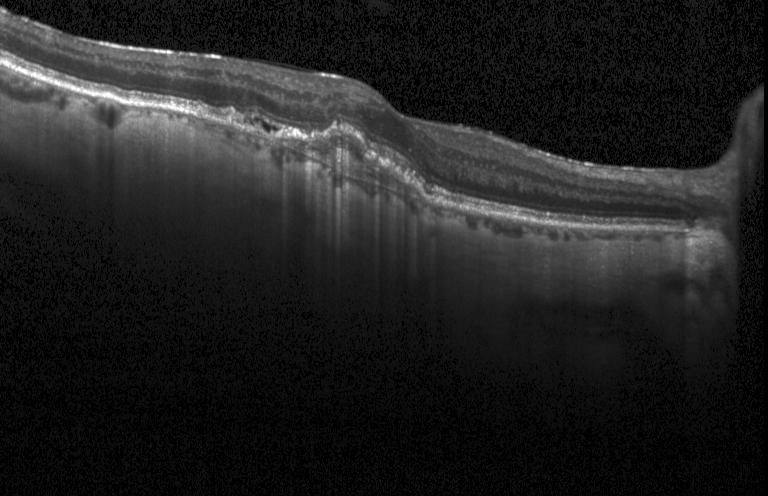

Optical coherence tomography scan; through the macula; spectral-domain OCT; Heidelberg Spectralis OCT system — This B-scan demonstrates choroidal neovascularization (CNV).